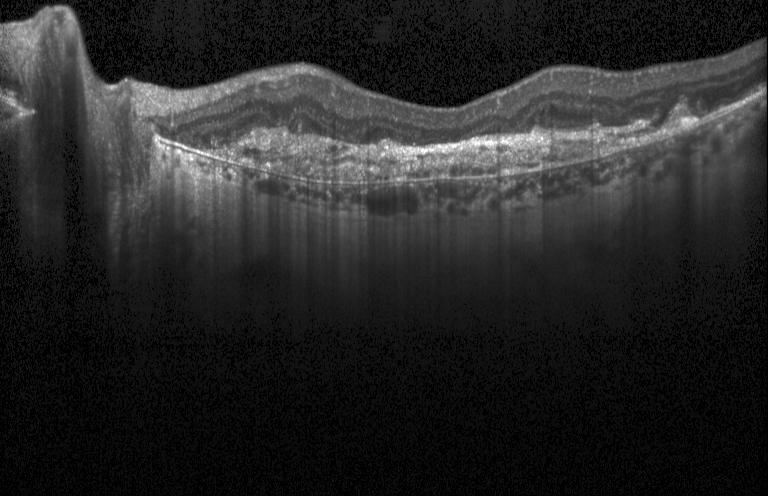
Heidelberg Spectralis OCT system · optical coherence tomography B-scan. Impression: choroidal neovascularization (CNV).